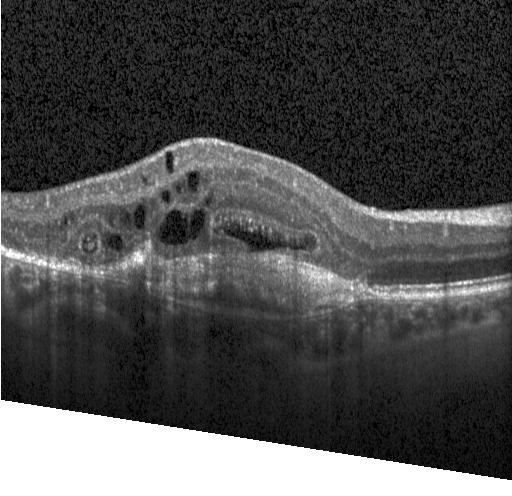 Optical coherence tomography scan; acquired on a Heidelberg Spectralis; spectral-domain OCT.
OCT finding: CNV.